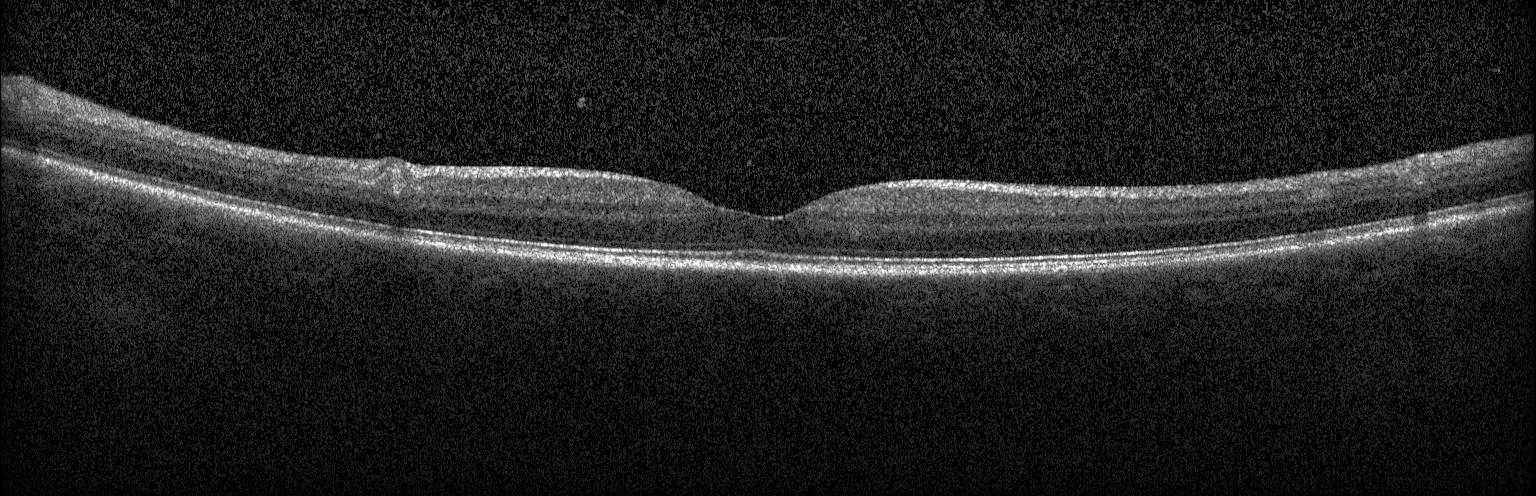 Retinal OCT B-scan; instrument: Heidelberg Spectralis
The scan shows no choroidal neovascularization, diabetic macular edema, or drusen.